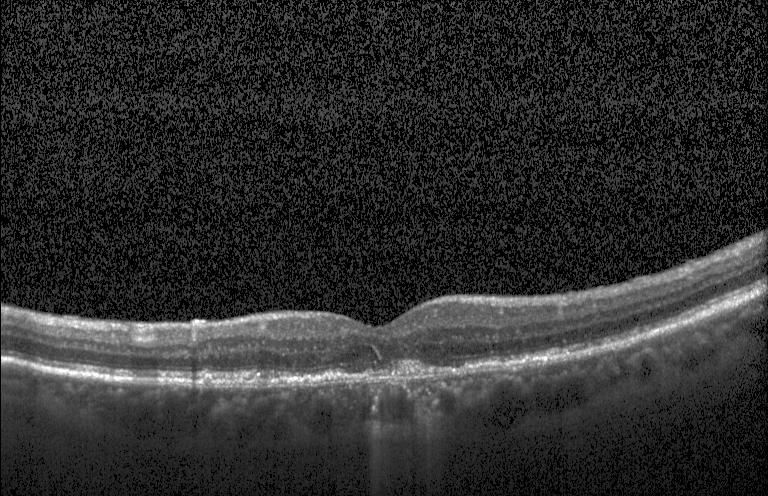 Optical coherence tomography B-scan · Heidelberg Spectralis OCT system · SD-OCT
This B-scan demonstrates choroidal neovascularization.